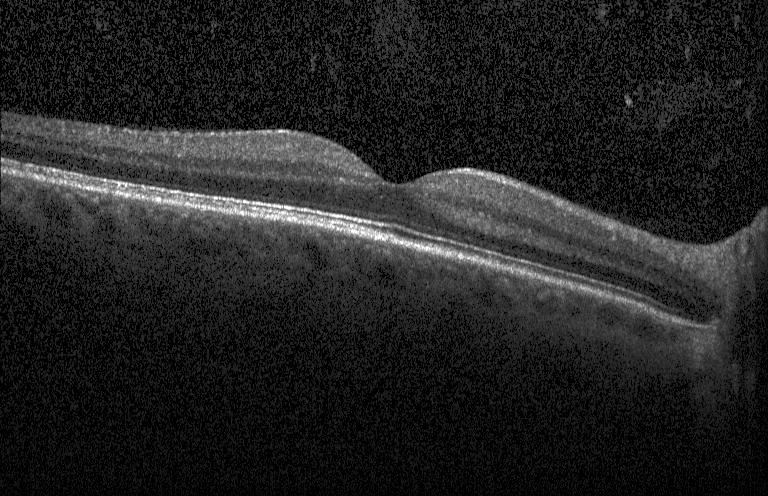

Diagnosis: no CNV, no DME, and no drusen.